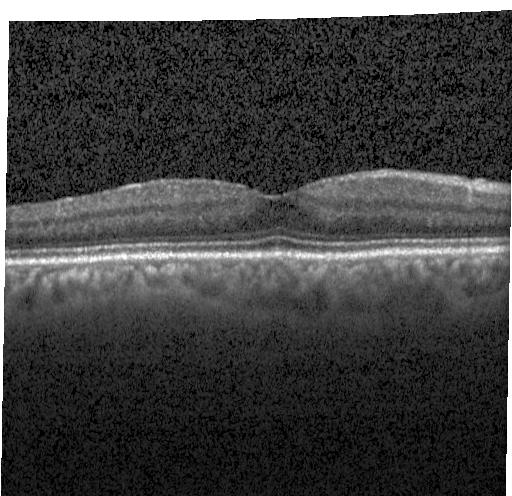
SD-OCT · OCT B-scan — Diagnosis: no choroidal neovascularization, diabetic macular edema, or drusen.